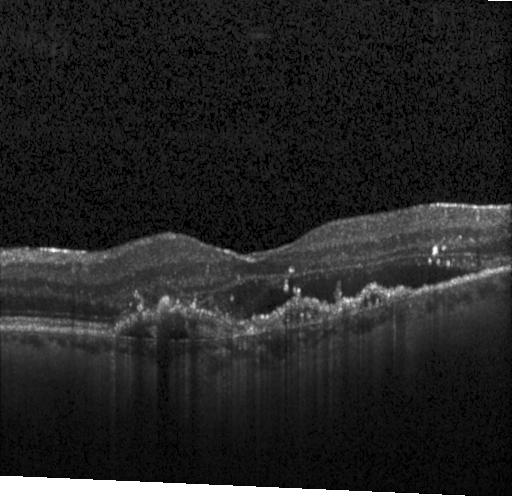
Retinal OCT cross-section · acquired on a Heidelberg Spectralis · through the macula. Assessment: choroidal neovascularization.